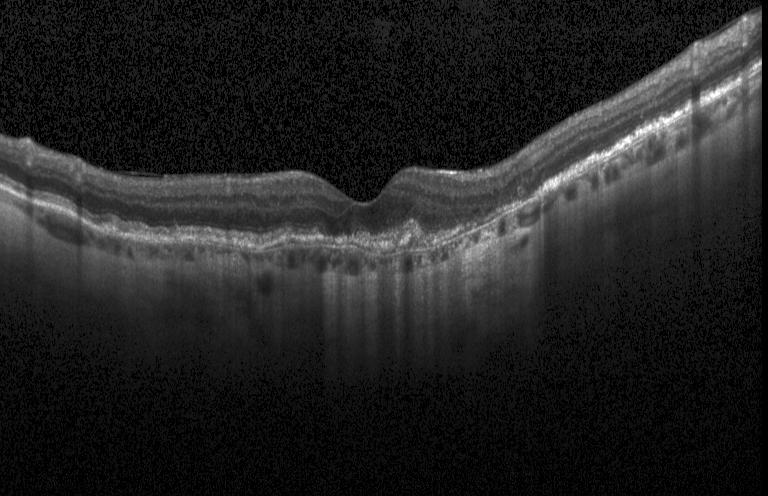 Finding: a choroidal neovascular membrane.